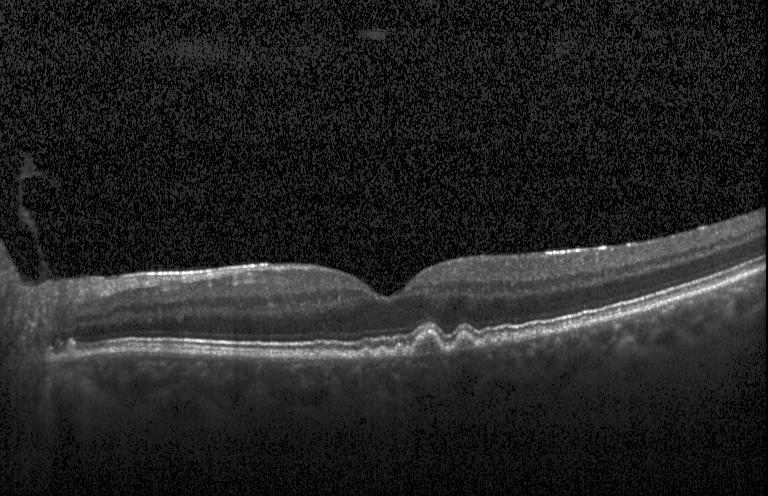
Retinal OCT cross-section, instrument: Heidelberg Spectralis, through the macula, spectral-domain optical coherence tomography
Diagnosis: sub-RPE drusenoid deposits.